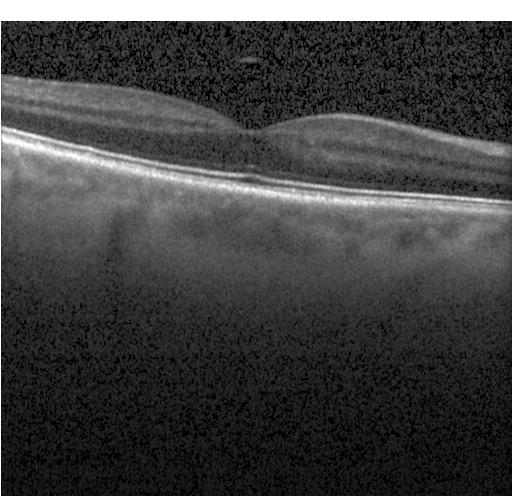

Macular OCT: no choroidal neovascularization, diabetic macular edema, or drusen.